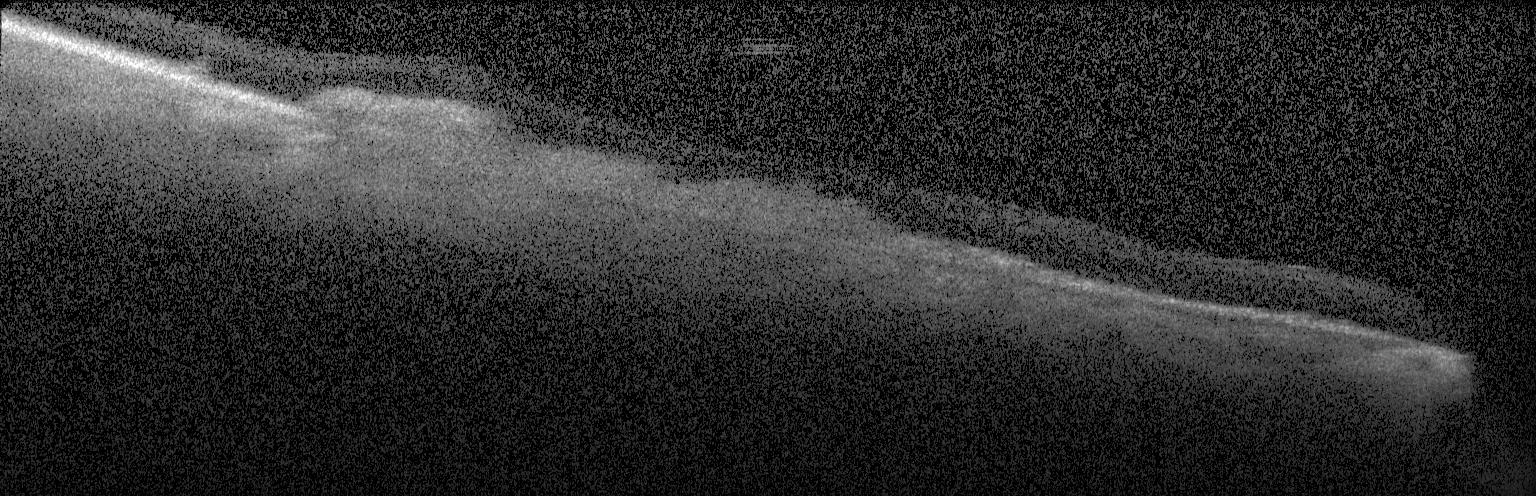 OCT line scan, spectral-domain OCT. Dx: CNV.